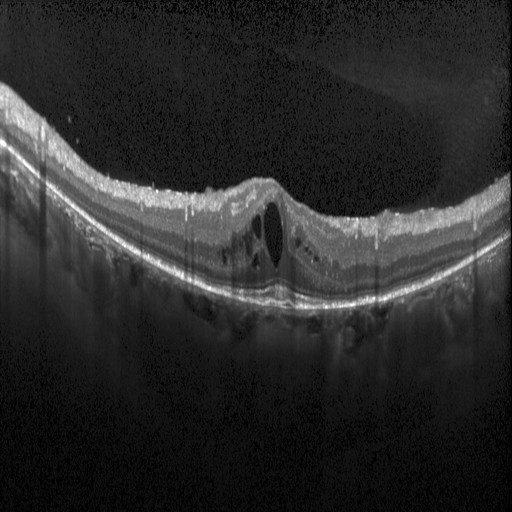

This B-scan demonstrates diabetic macular edema (DME).